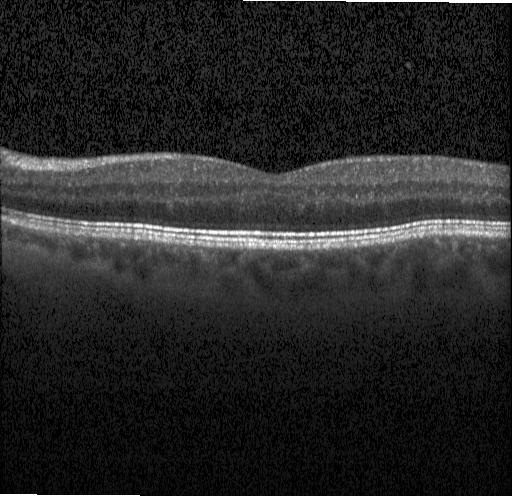
Optical coherence tomography B-scan. Horizontal scan through the fovea. SD-OCT. Acquired on a Heidelberg Spectralis.
Macular OCT: no CNV, DME, or drusen.